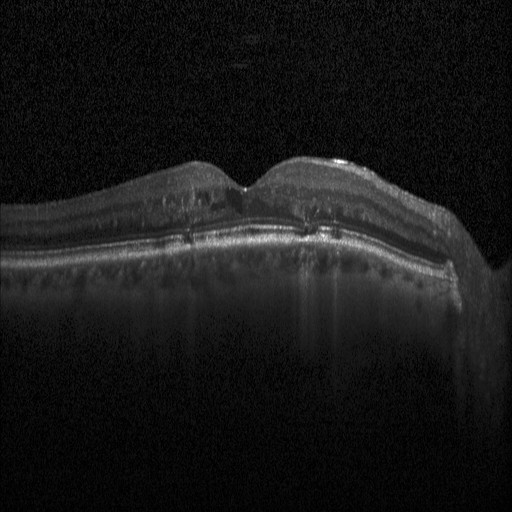

Impression: diabetic macular edema (DME).